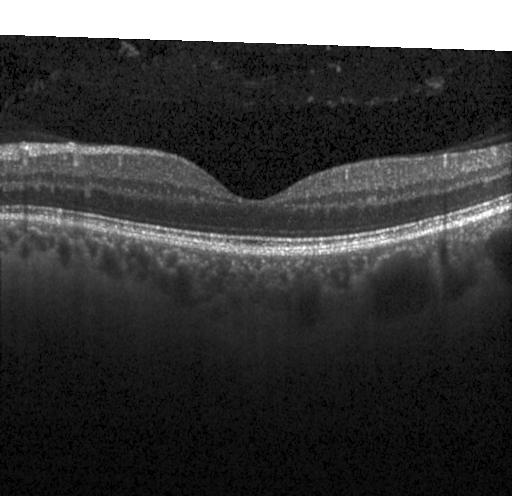
Dx: no choroidal neovascularization, diabetic macular edema, or drusen.